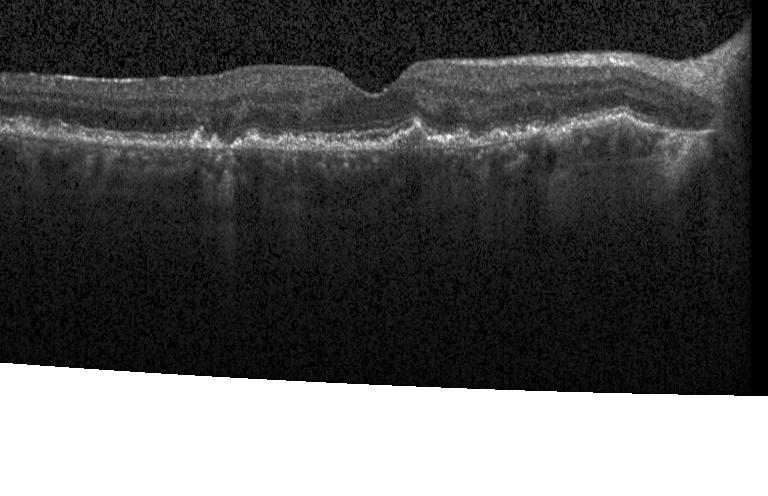 OCT finding: drusen.